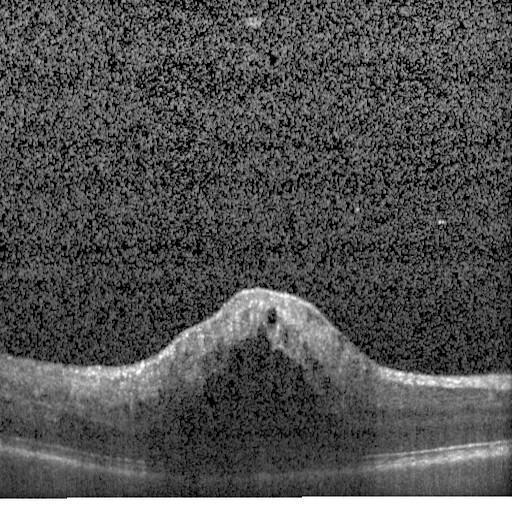

SD-OCT · instrument: Heidelberg Spectralis · optical coherence tomography scan · horizontal scan through the fovea
Macular OCT: DME.